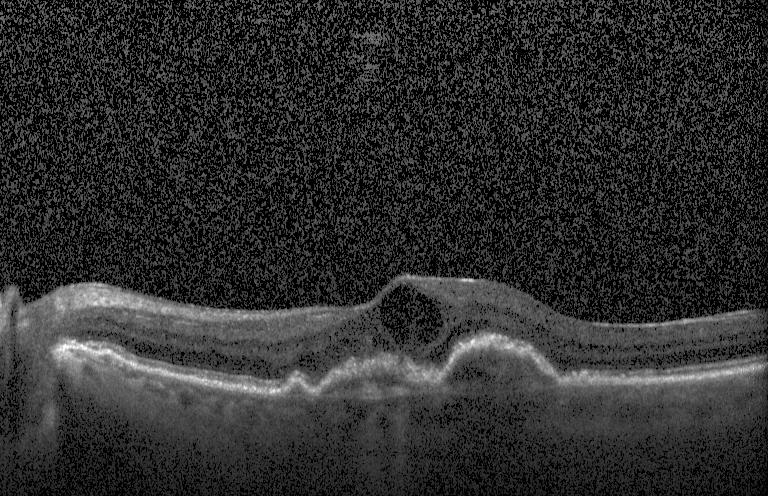

Optical coherence tomography B-scan. Horizontal scan through the fovea
Finding: CNV.